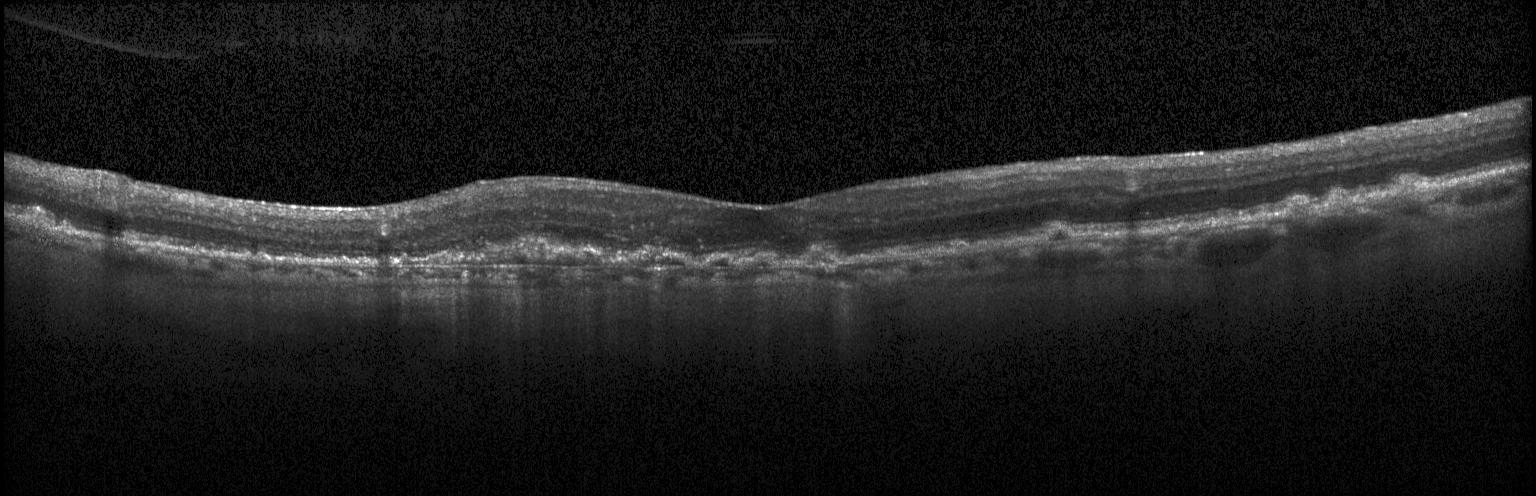
Macular OCT: choroidal neovascularization (CNV).